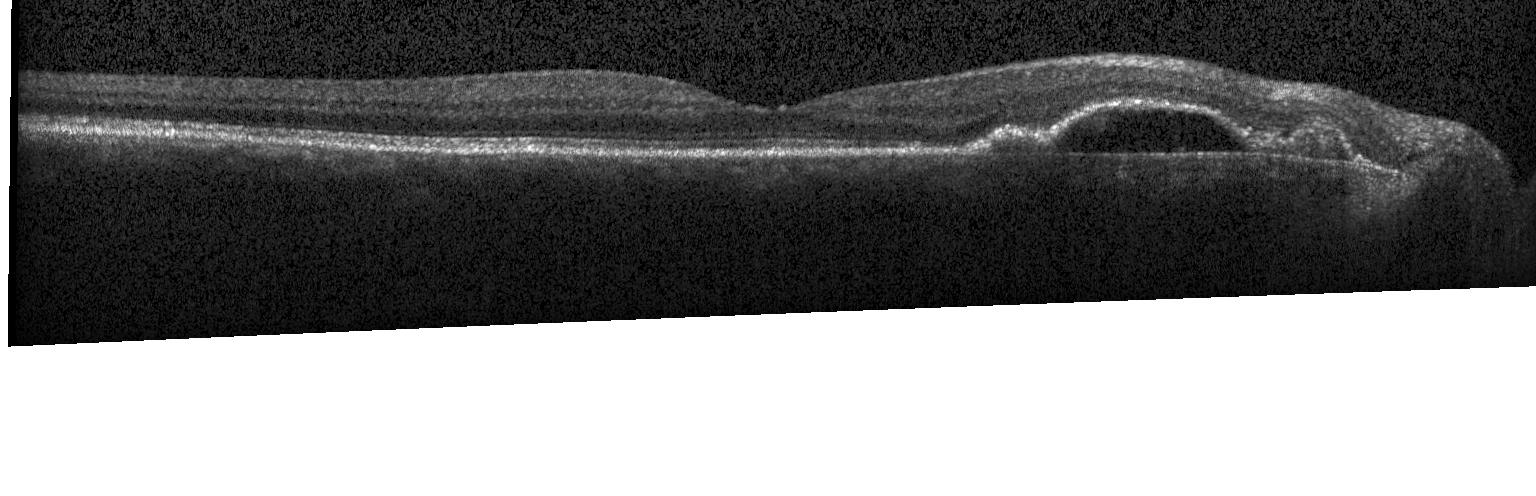 Optical coherence tomography scan.
Finding: choroidal neovascularization.